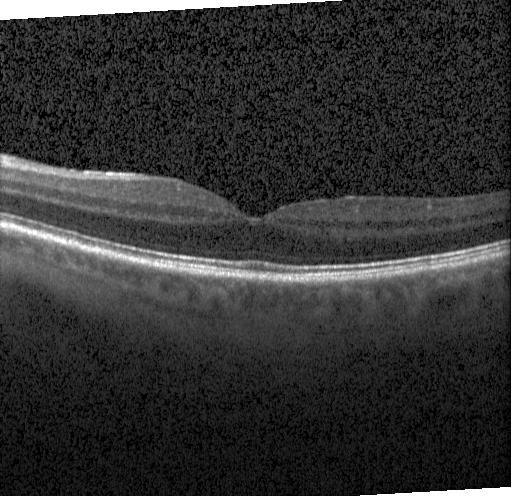

OCT scan showing no CNV, DME, or drusen.